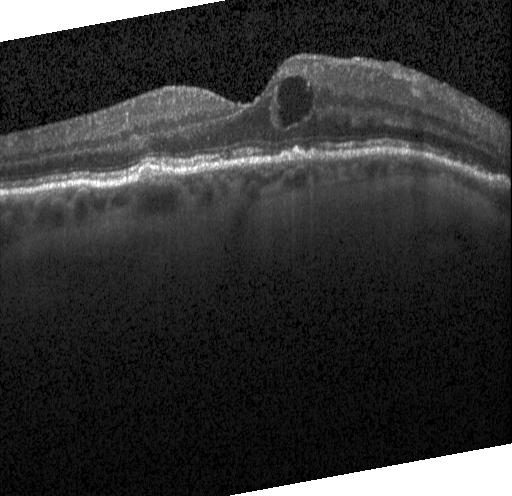

Centered on the fovea, OCT line scan
Diagnosis: a choroidal neovascular membrane.